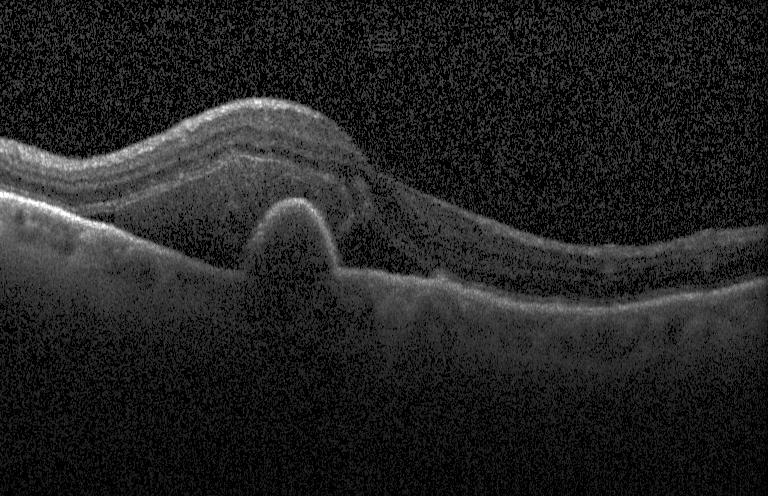
Retinal OCT B-scan.
Impression: choroidal neovascularization (CNV).